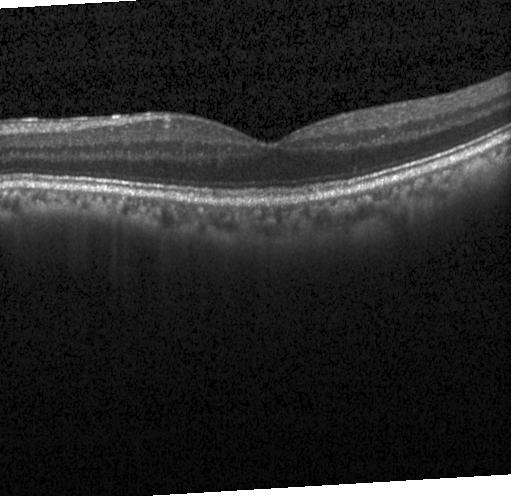 This B-scan demonstrates no choroidal neovascularization, no diabetic macular edema, and no drusen.